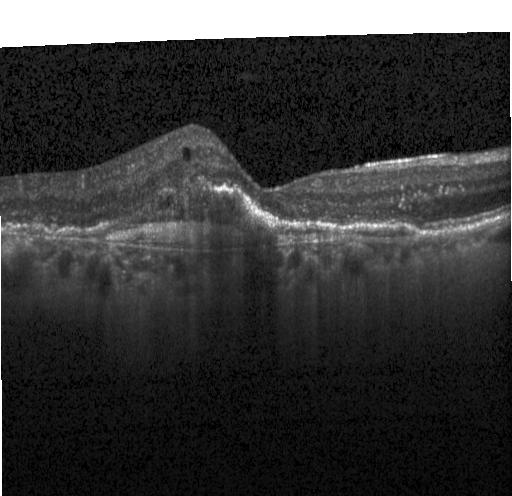

Heidelberg Spectralis; OCT B-scan; spectral-domain OCT. Impression: a choroidal neovascular membrane.